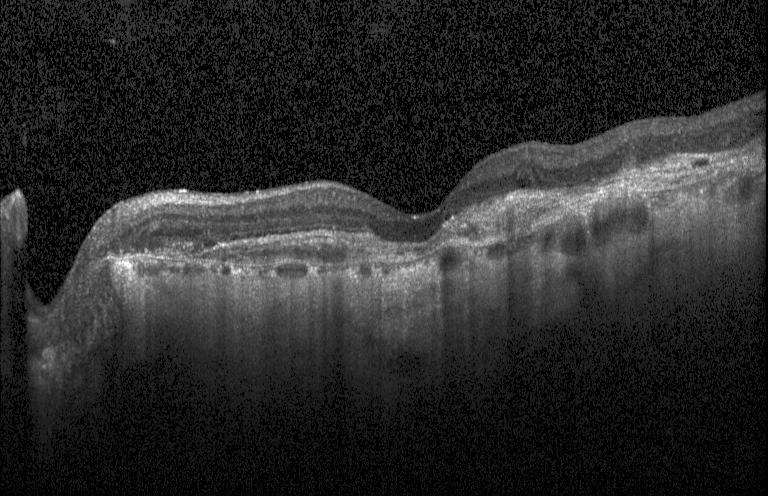 Horizontal scan through the fovea; Heidelberg Spectralis OCT system; optical coherence tomography B-scan
Macular OCT: a choroidal neovascular membrane.